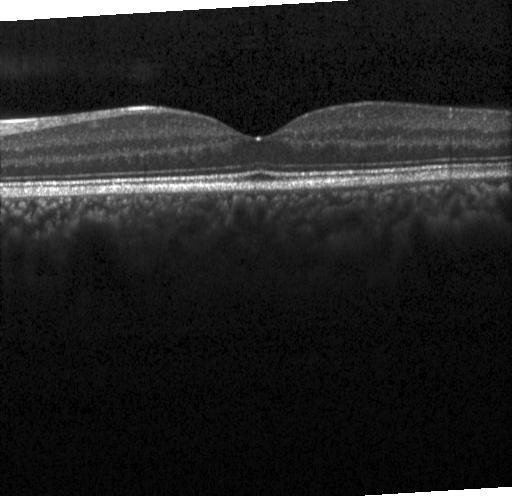

Dx: no CNV, no DME, and no drusen.